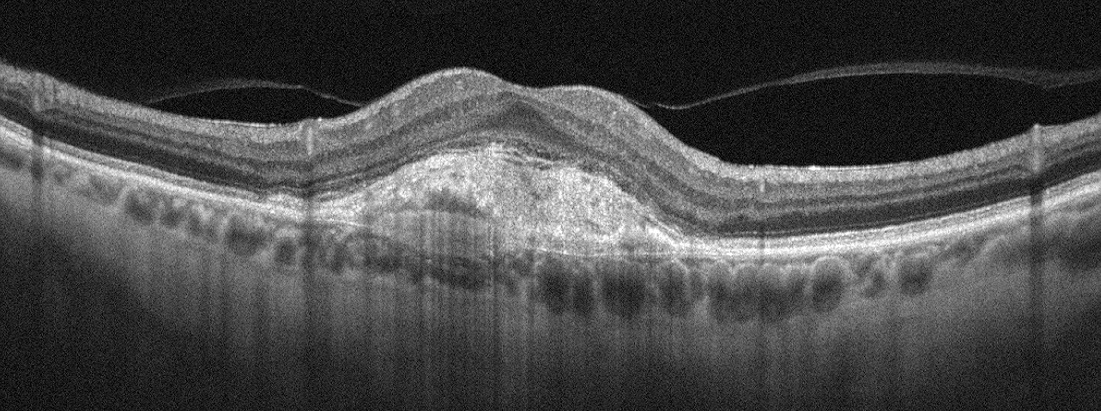
Impression: age-related macular degeneration.